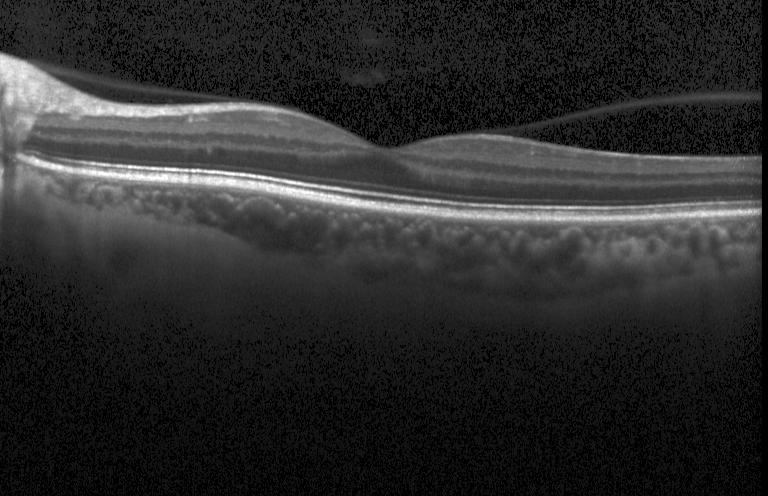
Macular OCT demonstrating no choroidal neovascularization, no diabetic macular edema, and no drusen.